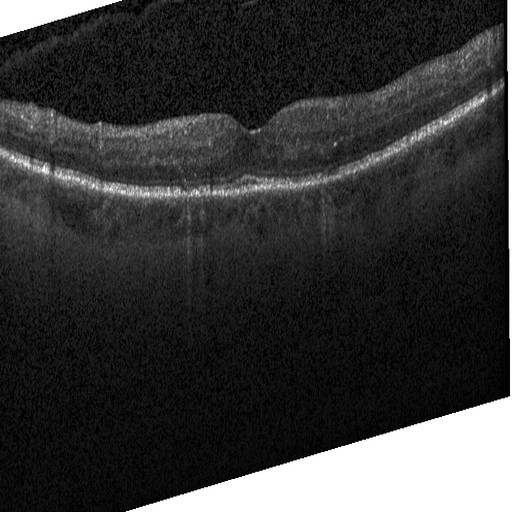

Optical coherence tomography B-scan
Diagnosis: diabetic macular edema (DME).